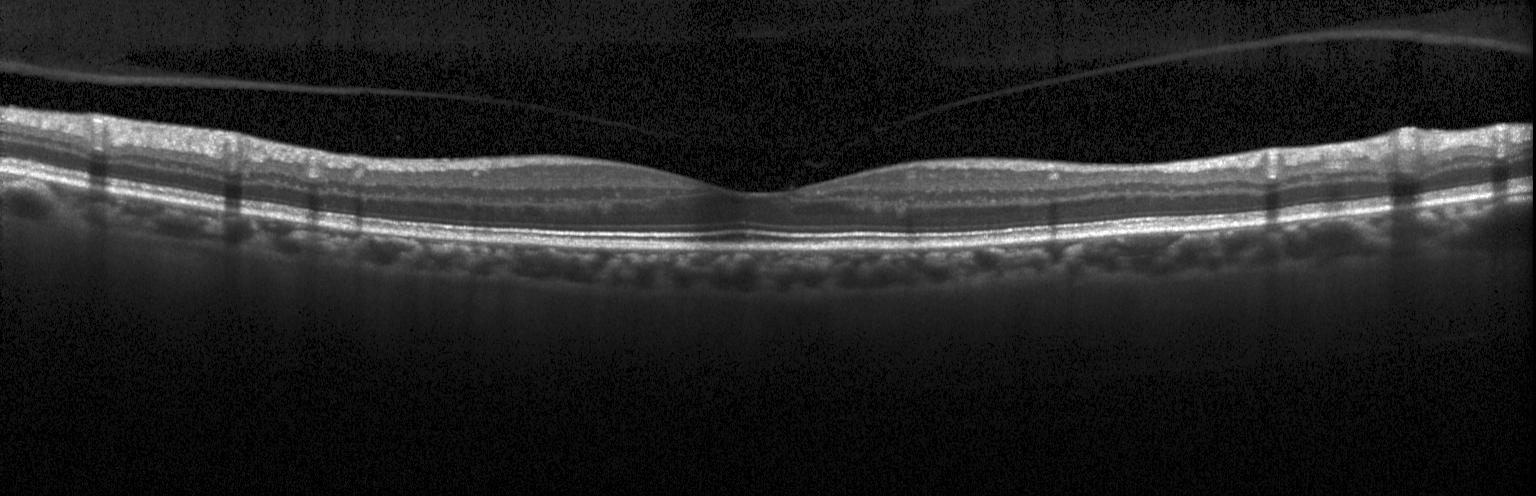

Spectral-domain OCT; OCT B-scan; macular scan; acquired on a Heidelberg Spectralis — Macular OCT: no evidence of CNV, DME, or drusen.